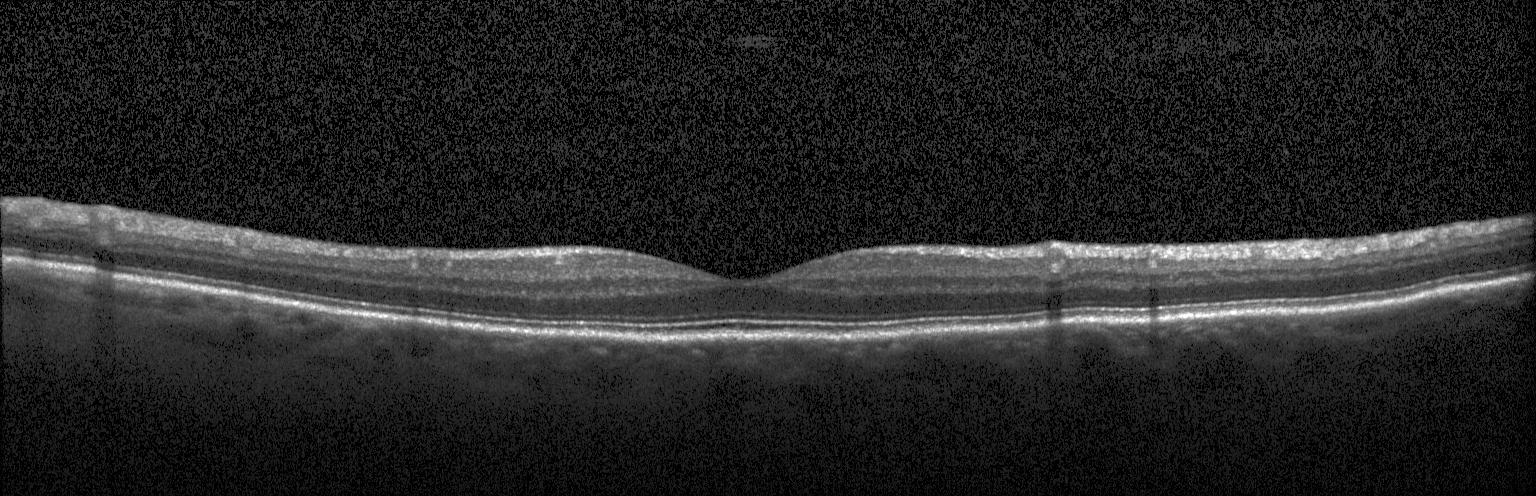

Retinal OCT B-scan. Macular scan. SD-OCT. Heidelberg Spectralis OCT system
OCT finding: no evidence of choroidal neovascularization, diabetic macular edema, or drusen.